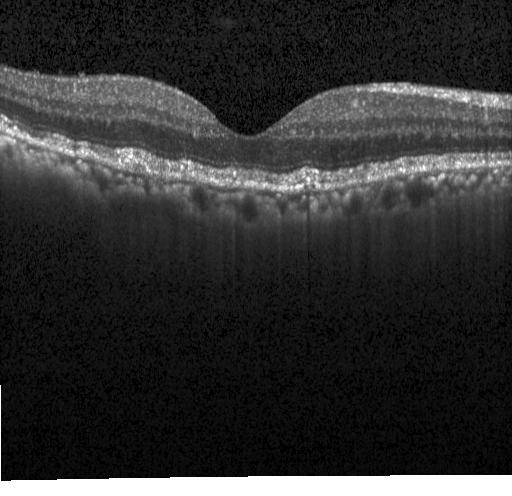

Finding: sub-RPE drusenoid deposits.